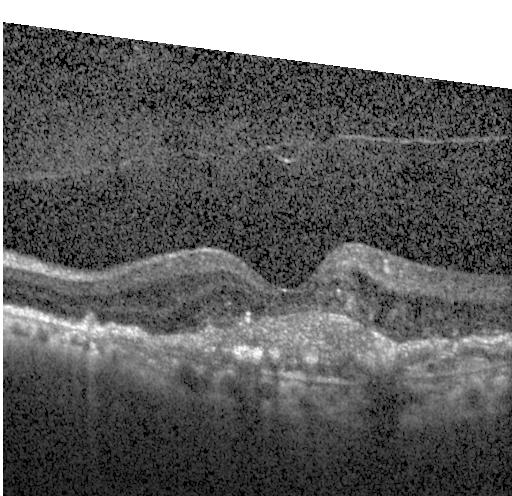
Macular scan · spectral-domain optical coherence tomography · acquired on a Heidelberg Spectralis · retinal OCT B-scan. Assessment: choroidal neovascularization (CNV).